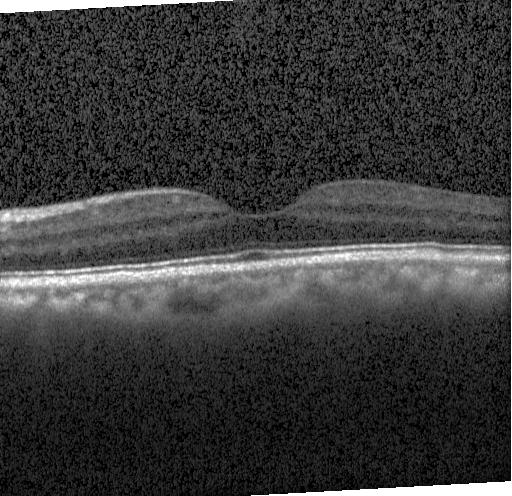 OCT scan showing no CNV, no DME, and no drusen.